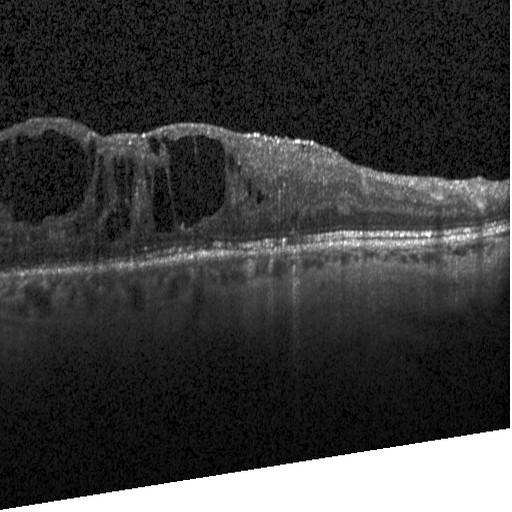 Impression: DME.